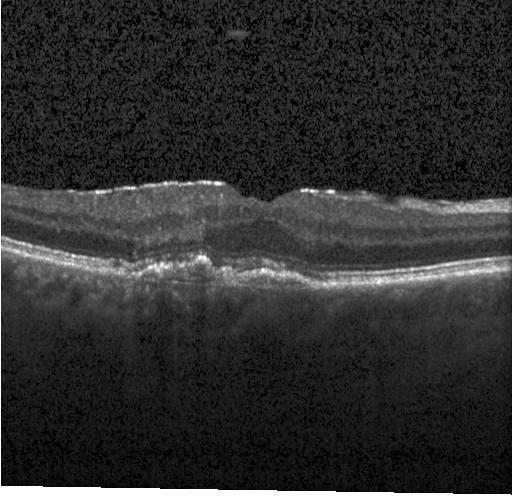 Retinal OCT B-scan
Finding: choroidal neovascularization.